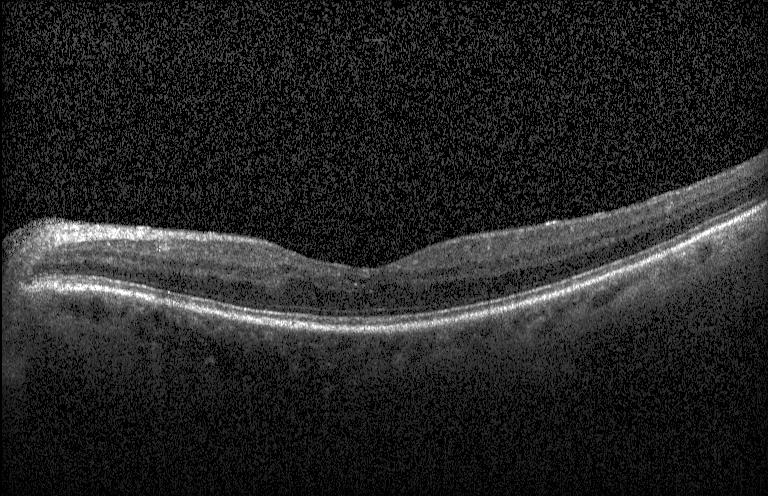

Fovea-centered. Optical coherence tomography B-scan. Instrument: Heidelberg Spectralis
Impression: no choroidal neovascularization, no diabetic macular edema, and no drusen.